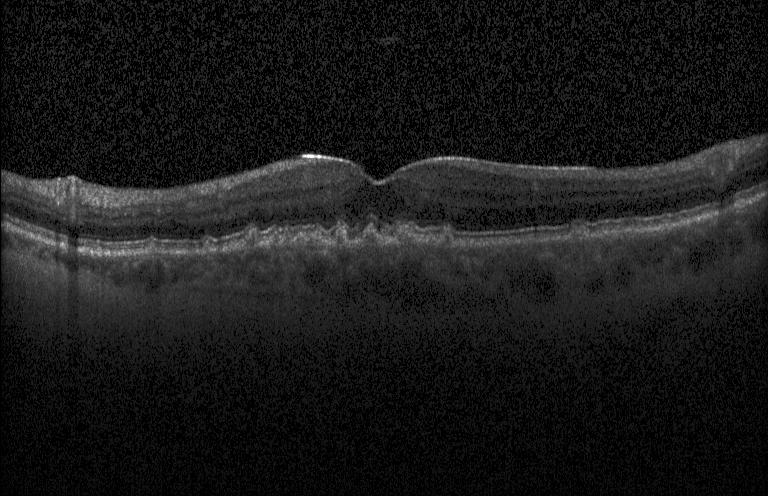
Finding: drusen.